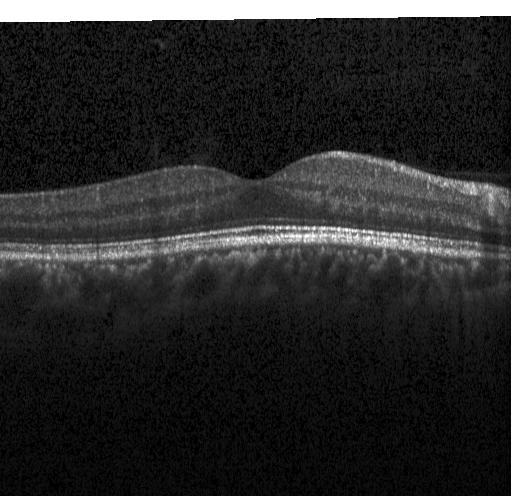

Heidelberg Spectralis OCT system. Retinal OCT B-scan — Assessment: no evidence of CNV, DME, or drusen.